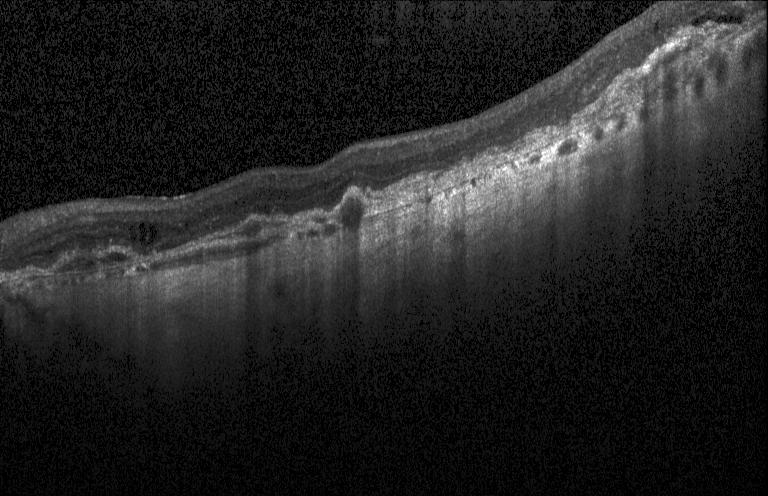
Horizontal scan through the fovea · optical coherence tomography B-scan — Impression: a choroidal neovascular membrane.